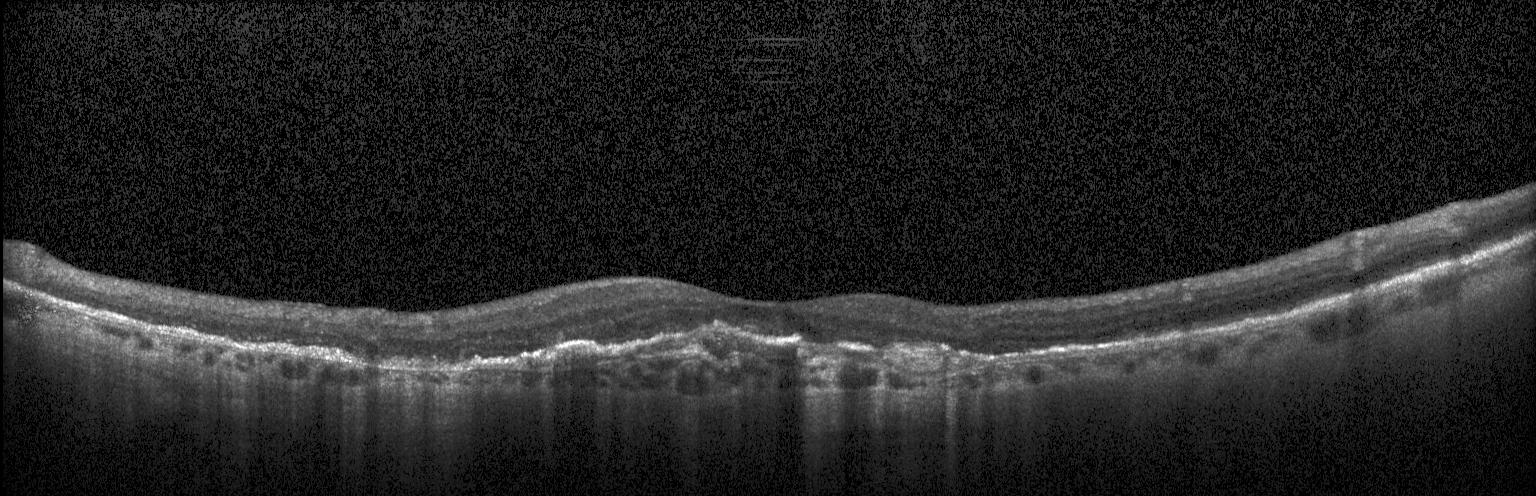 Macular OCT: CNV.